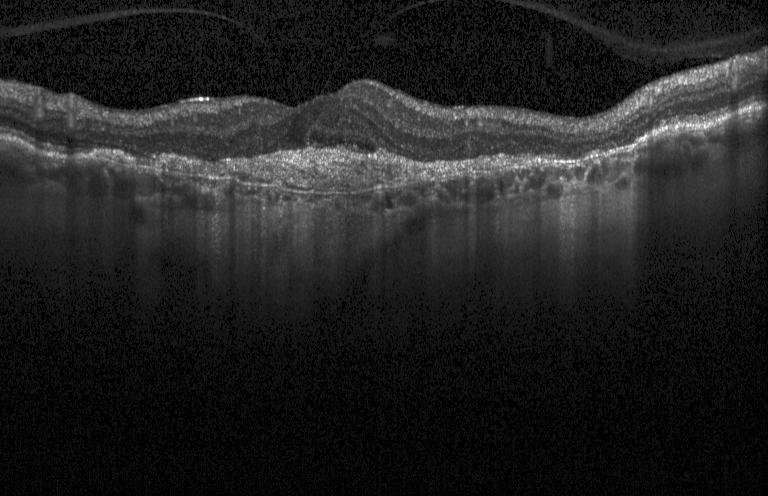

The scan shows a choroidal neovascular membrane.